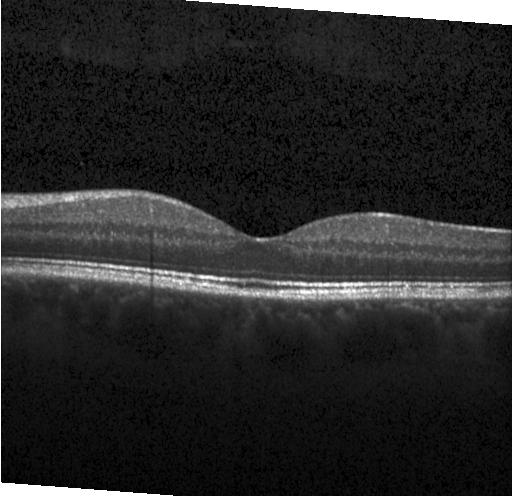

Fovea-centered, optical coherence tomography B-scan, SD-OCT, Heidelberg Spectralis
Diagnosis: neither choroidal neovascularization, diabetic macular edema, nor drusen.